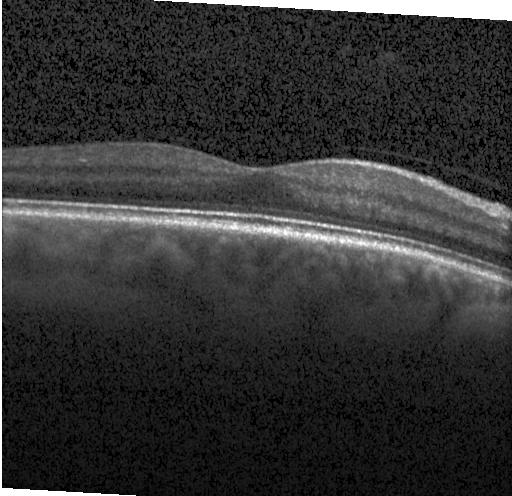

Assessment: no choroidal neovascularization, no diabetic macular edema, and no drusen.